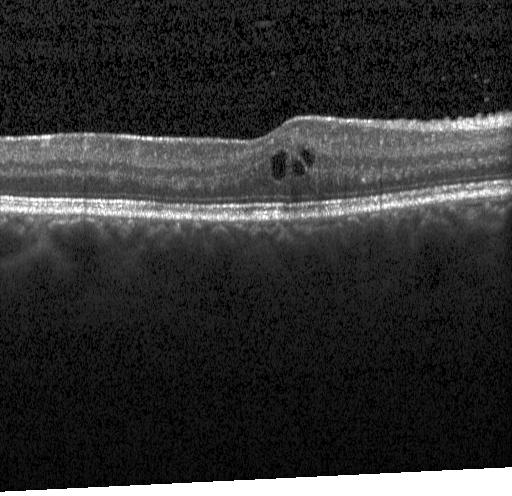

Finding: diabetic macular edema.